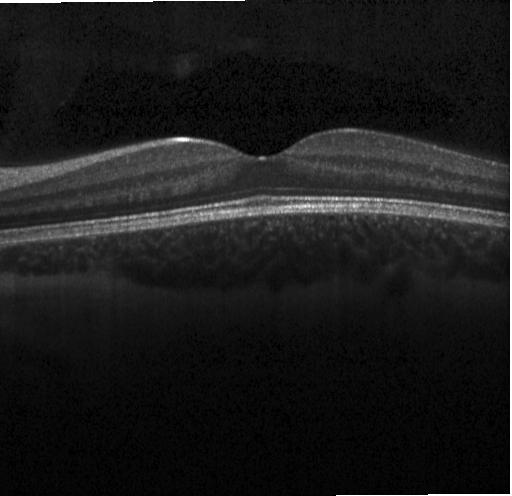 Retinal OCT cross-section.
Dx: neither choroidal neovascularization, diabetic macular edema, nor drusen.